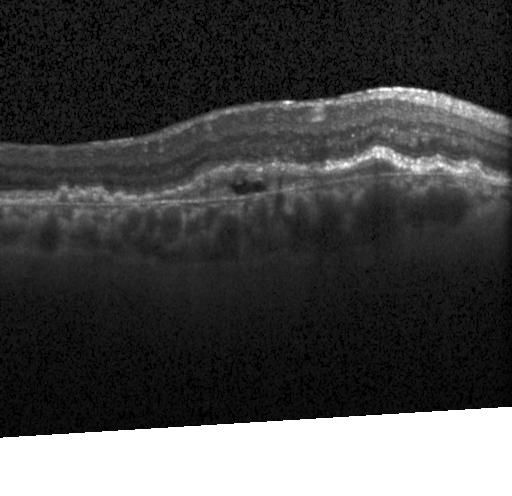 OCT B-scan; fovea-centered; instrument: Heidelberg Spectralis. Diagnosis: a choroidal neovascular membrane.